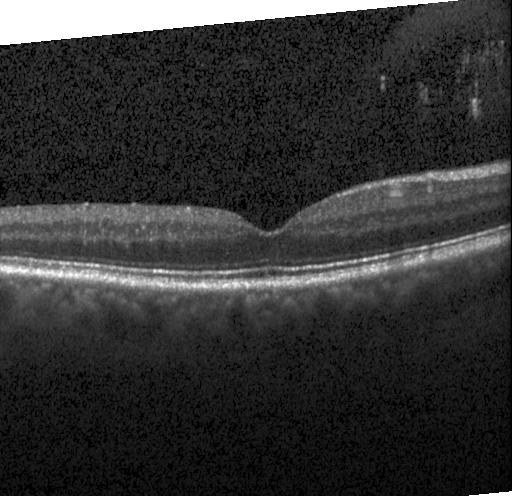 OCT finding: no choroidal neovascularization, diabetic macular edema, or drusen.